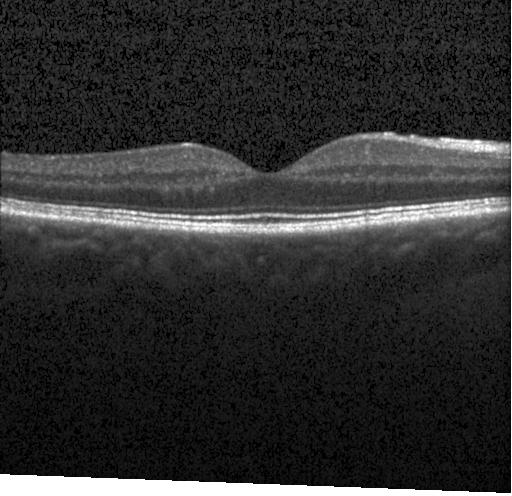 Acquired on a Heidelberg Spectralis, retinal OCT cross-section.
Dx: no choroidal neovascularization, diabetic macular edema, or drusen.